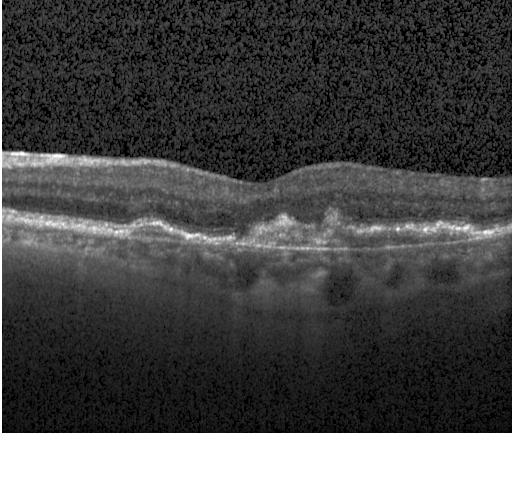
OCT line scan.
Impression: a choroidal neovascular membrane.